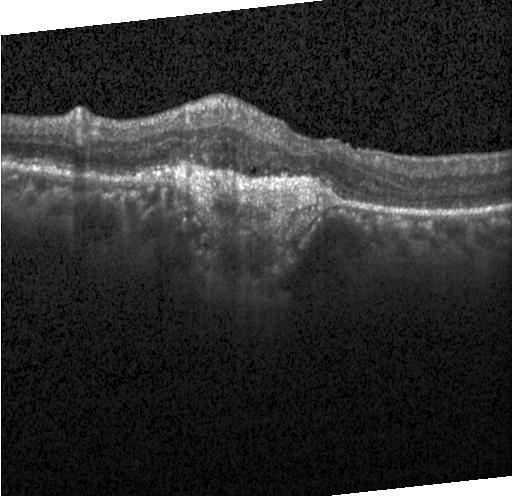
Retinal OCT cross-section
Assessment: CNV.